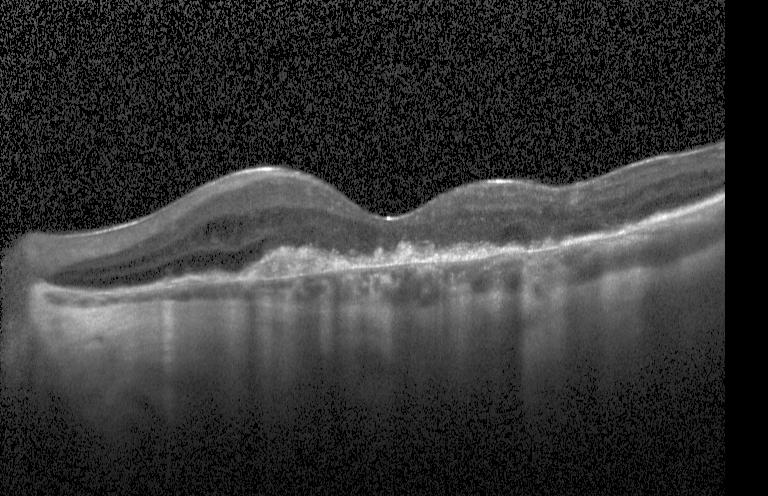

Impression: a choroidal neovascular membrane.